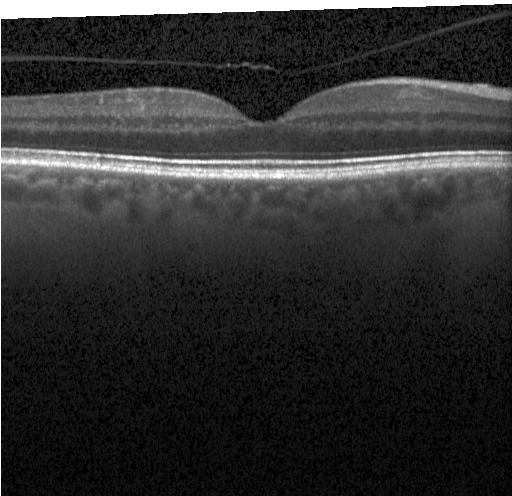
Optical coherence tomography scan. Centered on the fovea. SD-OCT. Instrument: Heidelberg Spectralis.
No choroidal neovascularization, no diabetic macular edema, and no drusen.